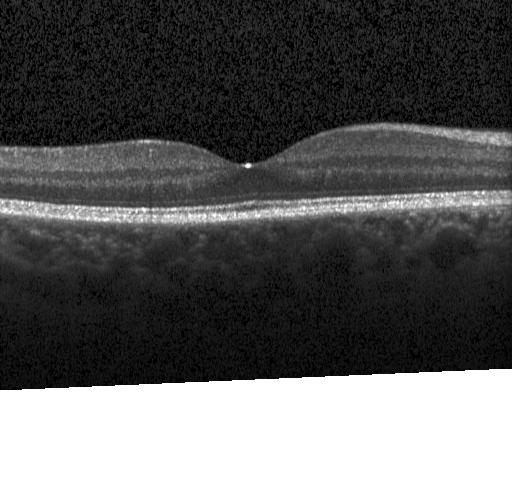 Retinal OCT cross-section. Macular scan. Assessment: no choroidal neovascularization, no diabetic macular edema, and no drusen.